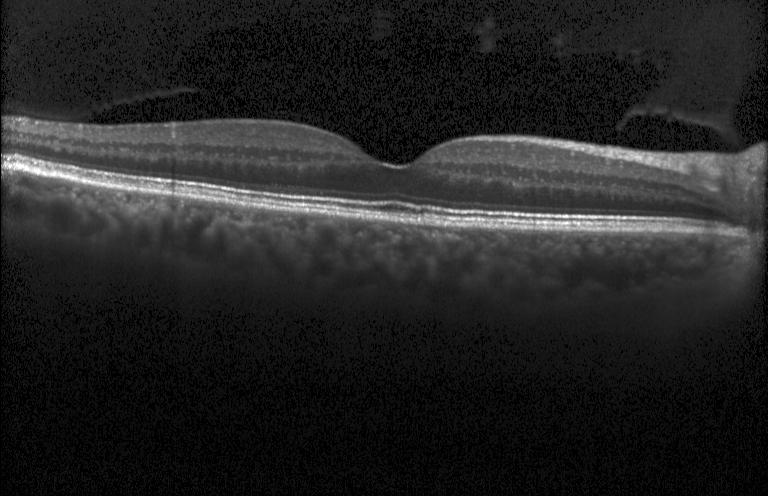
Acquired on a Heidelberg Spectralis, spectral-domain OCT, OCT B-scan, horizontal scan through the fovea. Impression: neither choroidal neovascularization, diabetic macular edema, nor drusen.